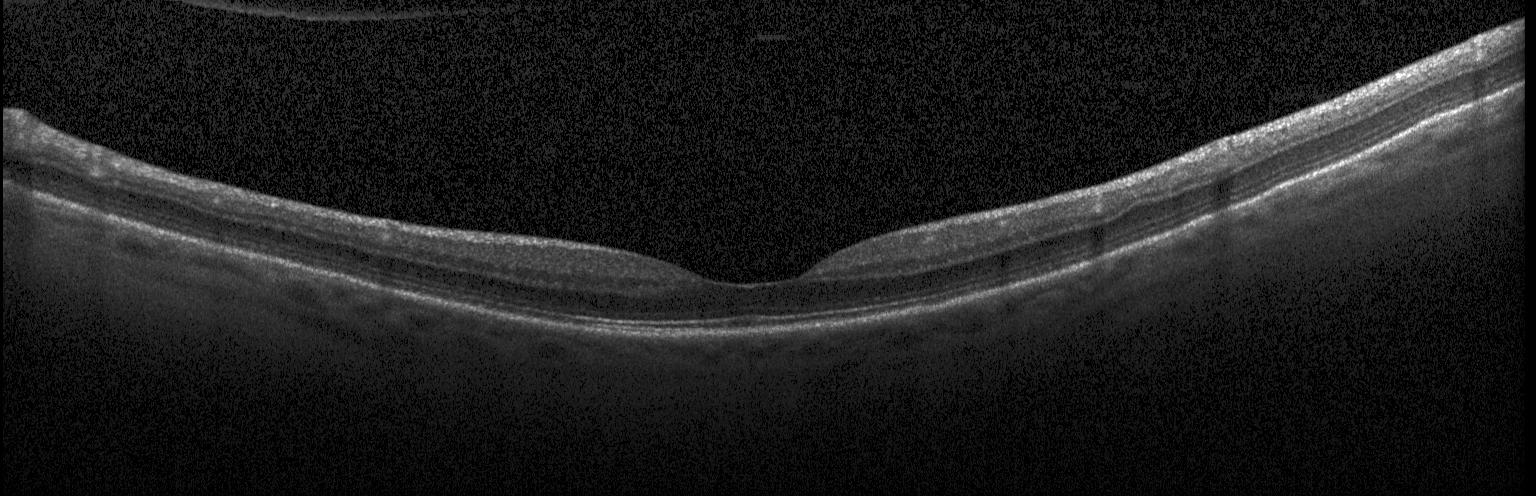

SD-OCT, retinal OCT cross-section — Dx: no evidence of choroidal neovascularization, diabetic macular edema, or drusen.